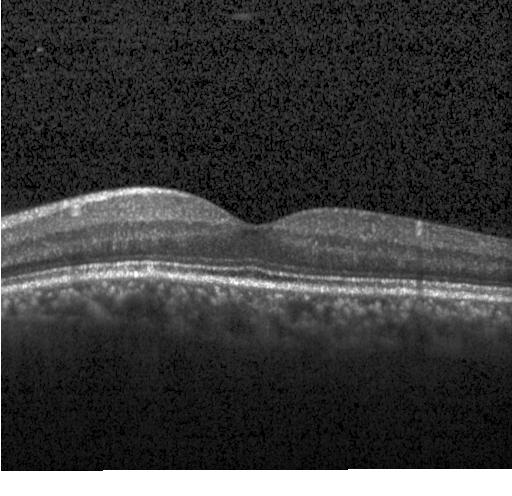 Spectral-domain optical coherence tomography; retinal OCT B-scan; instrument: Heidelberg Spectralis; horizontal scan through the fovea.
Impression: no CNV, DME, or drusen.